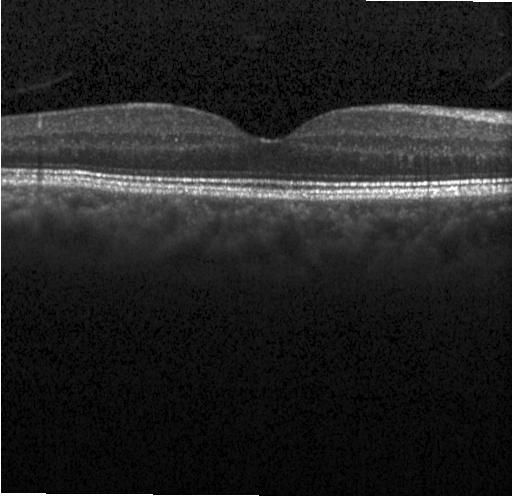
OCT line scan
Assessment: no CNV, DME, or drusen.